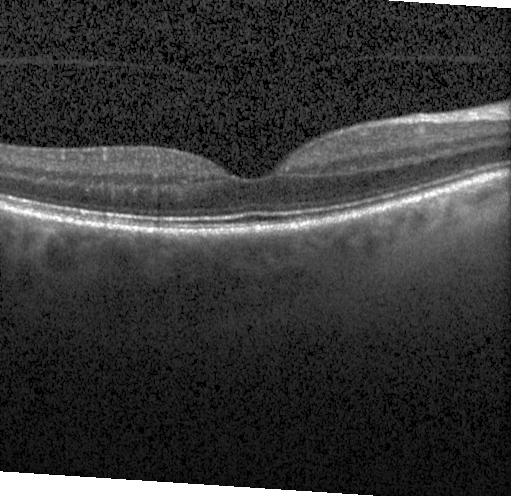
Assessment: no CNV, no DME, and no drusen.